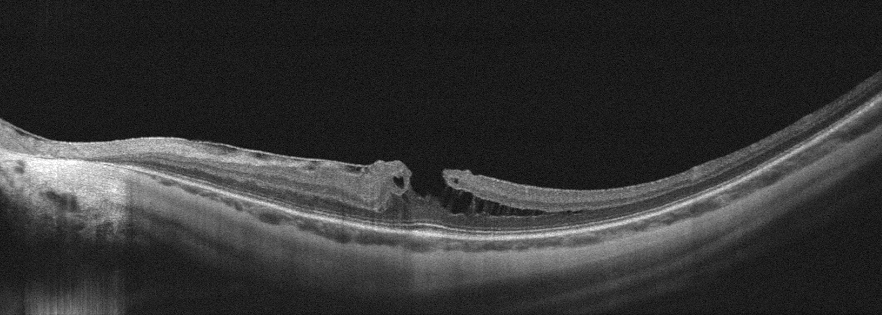

OS; OCT line scan
This B-scan demonstrates vitreomacular interface disease (VID).